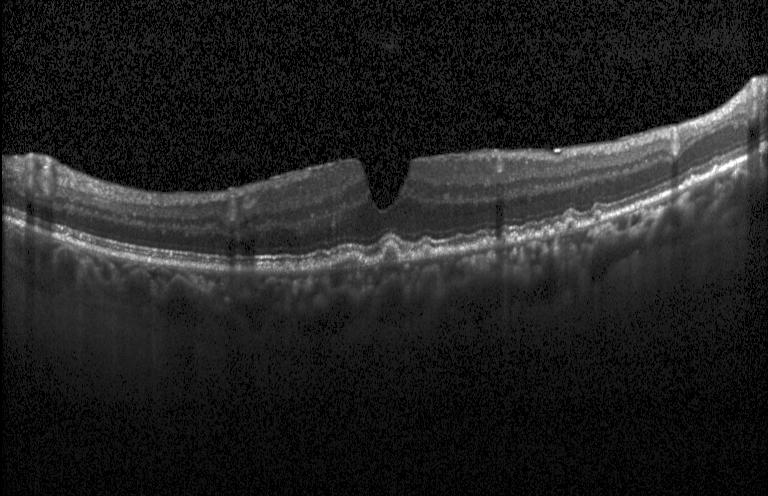
Heidelberg Spectralis. Macular scan. Spectral-domain OCT. Optical coherence tomography B-scan — Multiple drusen.